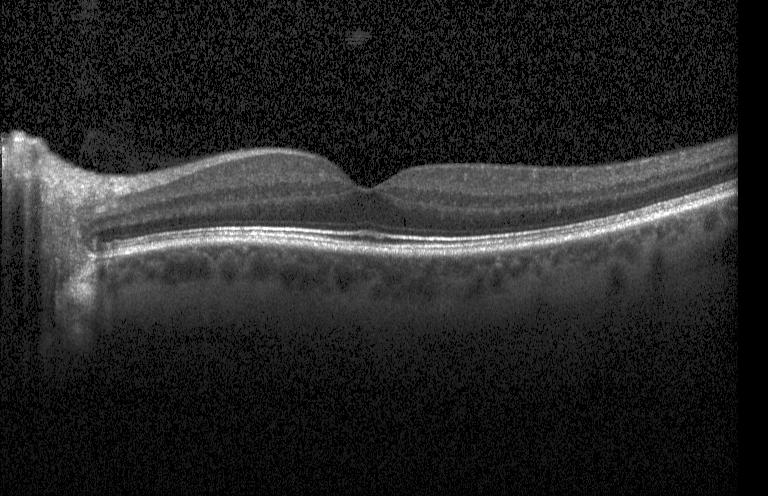 Optical coherence tomography scan, macular scan
Dx: no choroidal neovascularization, no diabetic macular edema, and no drusen.